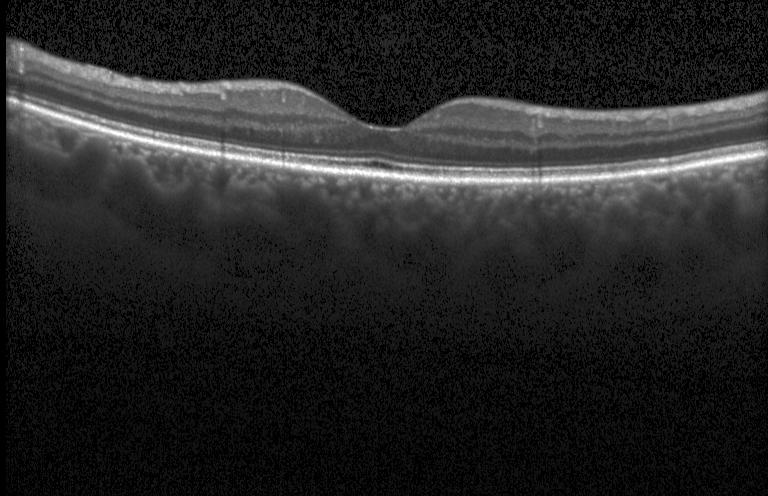
Spectral-domain OCT, instrument: Heidelberg Spectralis, fovea-centered, retinal OCT B-scan.
Finding: no choroidal neovascularization, no diabetic macular edema, and no drusen.